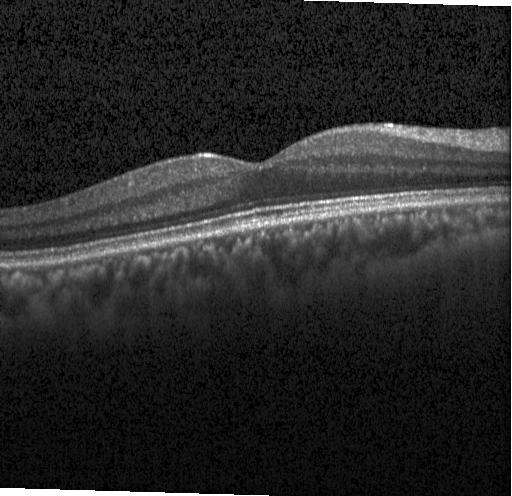
Spectral-domain OCT; centered on the fovea; OCT line scan; Heidelberg Spectralis OCT system — Assessment: no choroidal neovascularization, diabetic macular edema, or drusen.